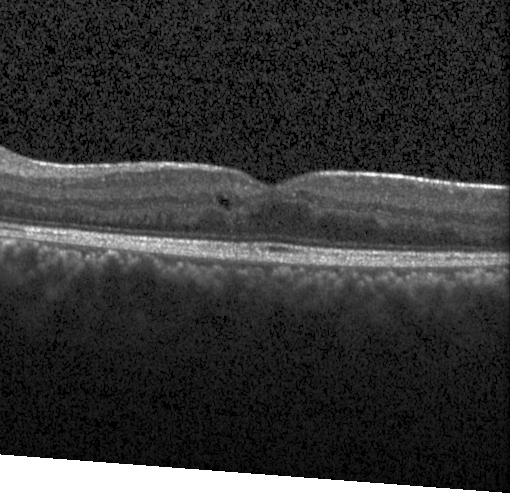 Retinal OCT B-scan. Acquired on a Heidelberg Spectralis. Centered on the fovea — Assessment: diabetic macular edema.